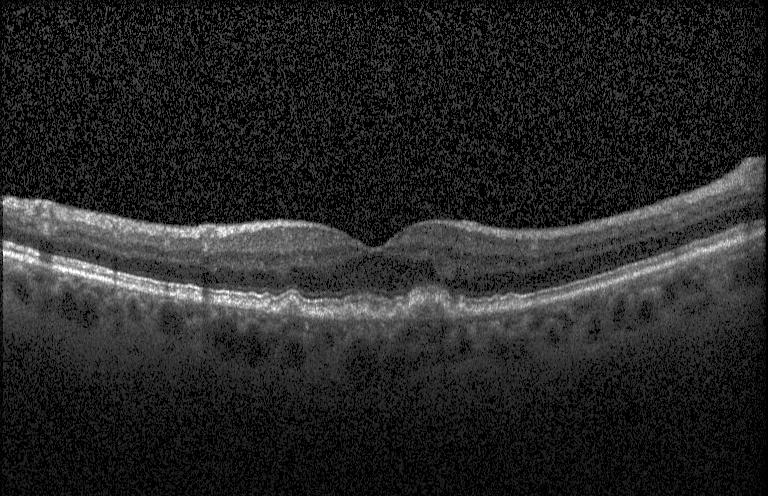 OCT B-scan. Multiple drusen.